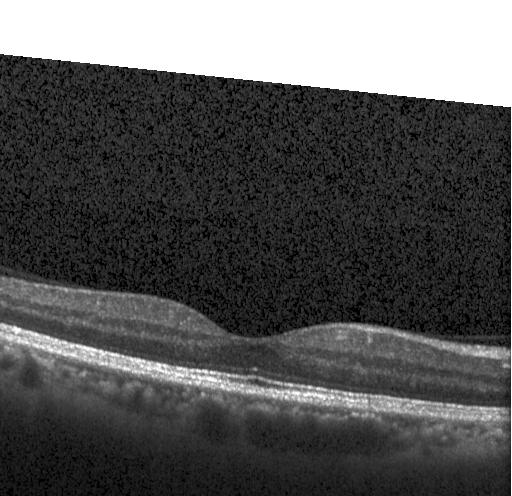 Centered on the fovea · OCT line scan · spectral-domain optical coherence tomography · Heidelberg Spectralis — Macular OCT: neither choroidal neovascularization, diabetic macular edema, nor drusen.